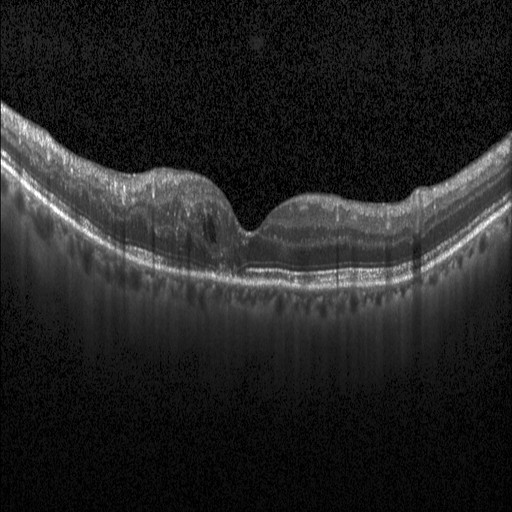

Acquired on a Heidelberg Spectralis; fovea-centered; OCT line scan
Finding: diabetic macular edema.